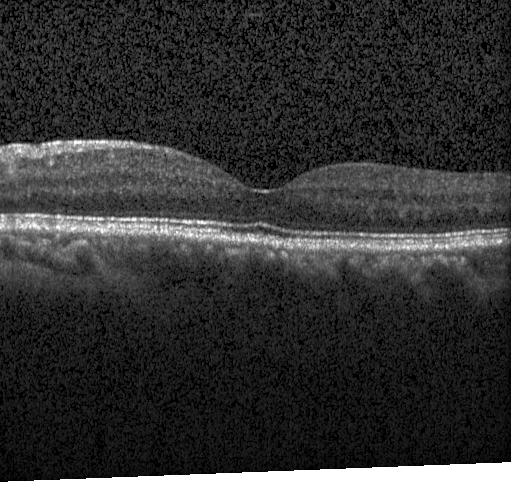

Finding: no choroidal neovascularization, no diabetic macular edema, and no drusen.